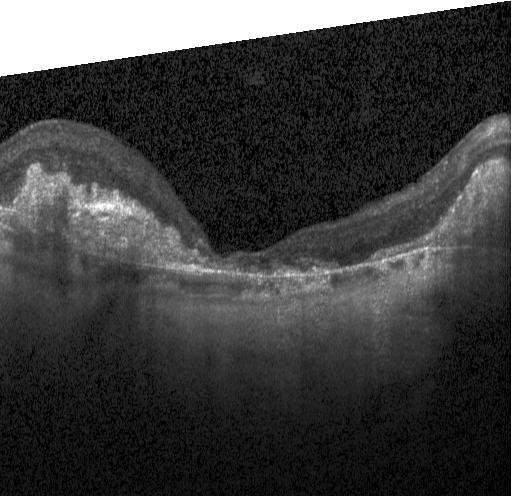

Spectral-domain OCT B-scan: a choroidal neovascular membrane.